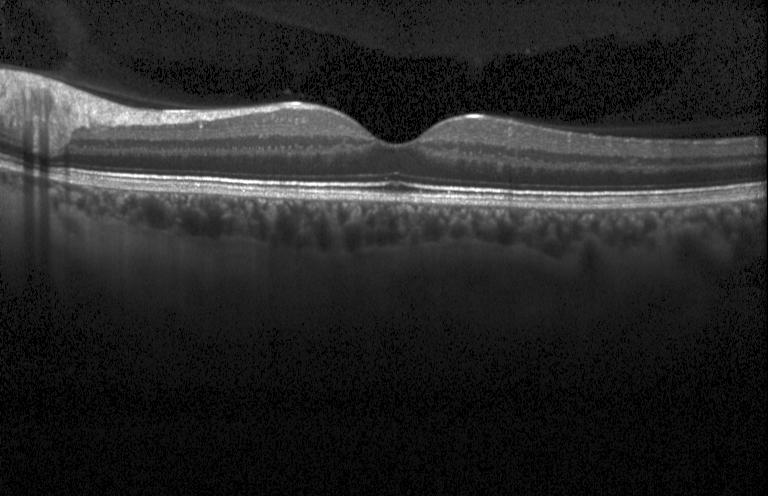

Retinal OCT B-scan.
Dx: no CNV, DME, or drusen.